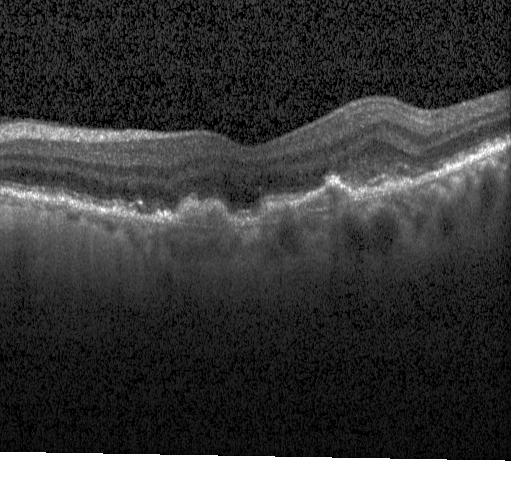 Fovea-centered, Heidelberg Spectralis, retinal OCT cross-section — Dx: choroidal neovascularization (CNV).